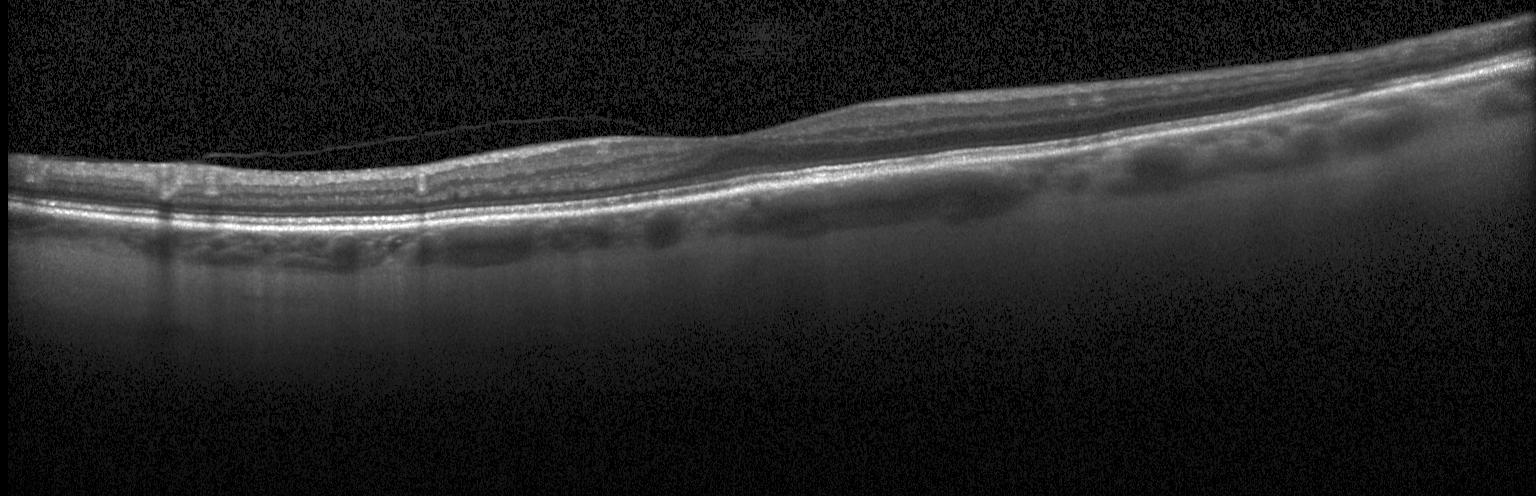 OCT B-scan. SD-OCT. Through the macula
Finding: no choroidal neovascularization, diabetic macular edema, or drusen.